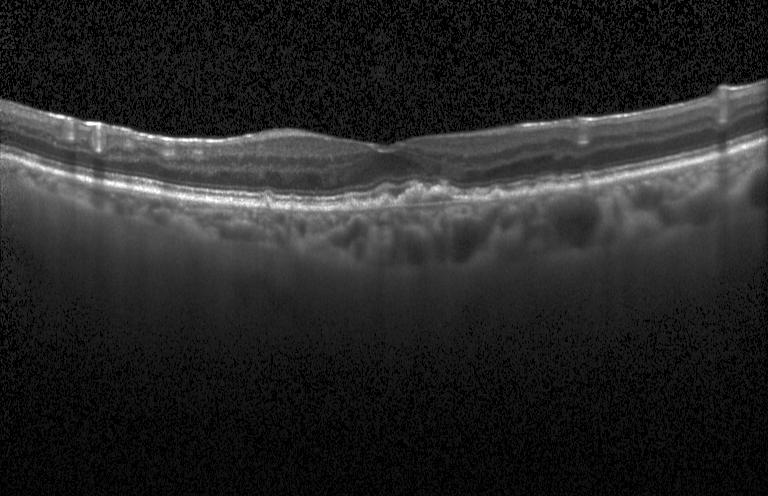
This B-scan demonstrates sub-RPE drusenoid deposits.